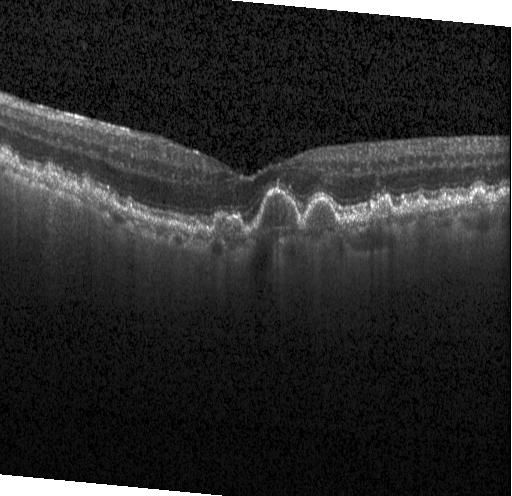
Macular OCT: sub-RPE drusenoid deposits.